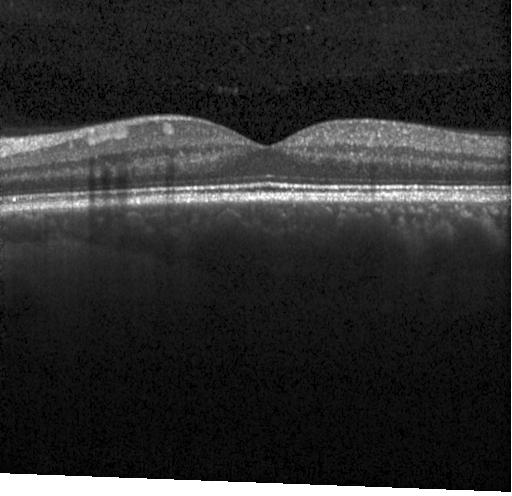

Acquired on a Heidelberg Spectralis, optical coherence tomography B-scan, horizontal scan through the fovea. This B-scan demonstrates neither choroidal neovascularization, diabetic macular edema, nor drusen.